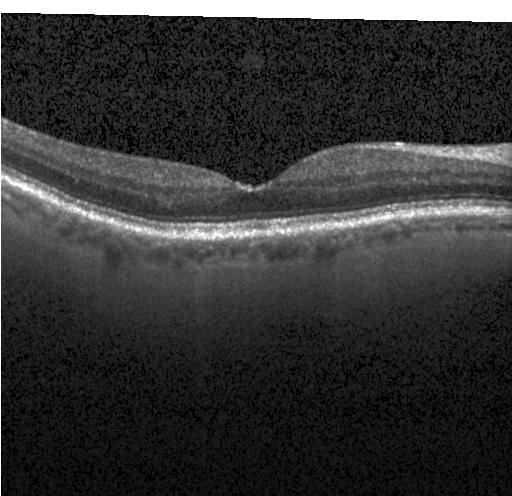

Spectral-domain optical coherence tomography; retinal OCT B-scan
Macular OCT: no evidence of choroidal neovascularization, diabetic macular edema, or drusen.